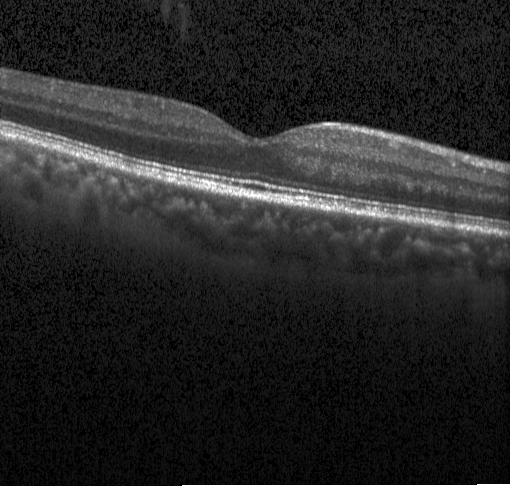

Impression: neither choroidal neovascularization, diabetic macular edema, nor drusen.